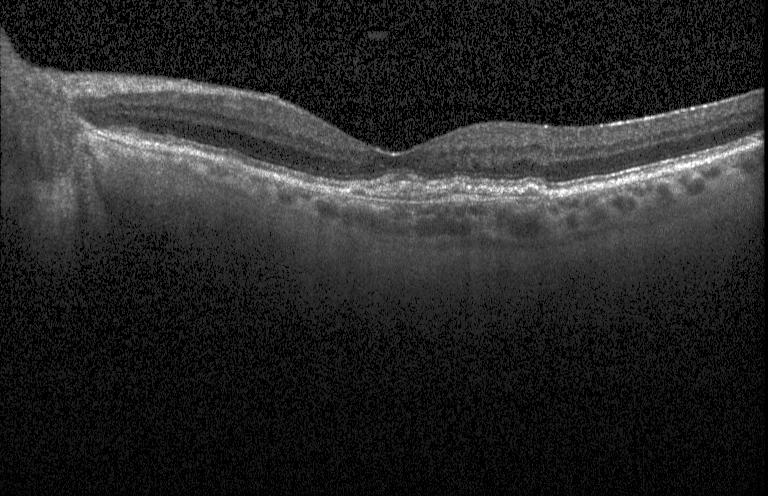

Retinal OCT cross-section
Diagnosis: CNV.